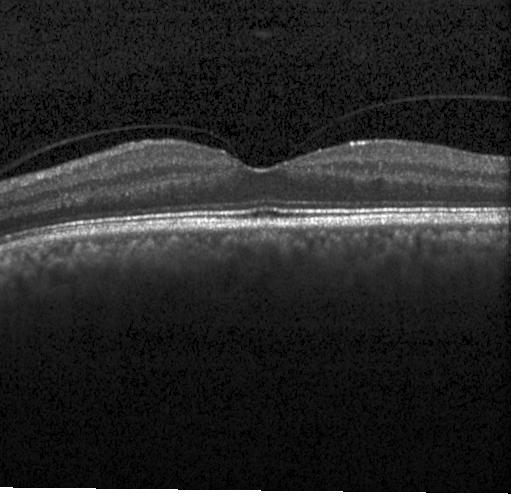 Finding: neither choroidal neovascularization, diabetic macular edema, nor drusen.